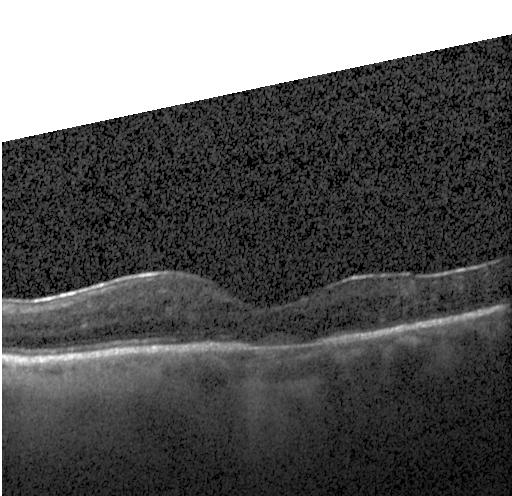 SD-OCT · optical coherence tomography scan · acquired on a Heidelberg Spectralis
This B-scan demonstrates a choroidal neovascular membrane.